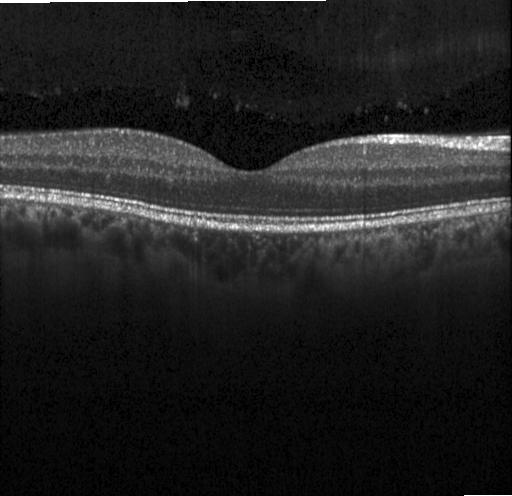

Macular scan, optical coherence tomography B-scan. Impression: no choroidal neovascularization, no diabetic macular edema, and no drusen.